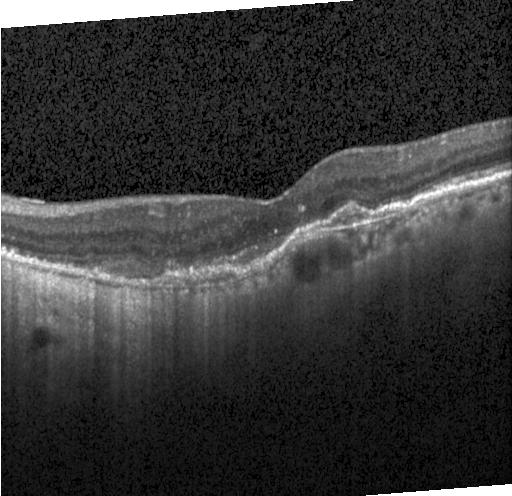 Retinal OCT B-scan — Assessment: choroidal neovascularization (CNV).